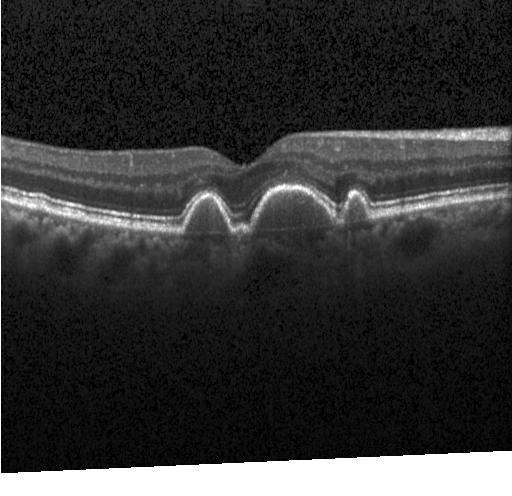 OCT finding: sub-RPE drusenoid deposits.